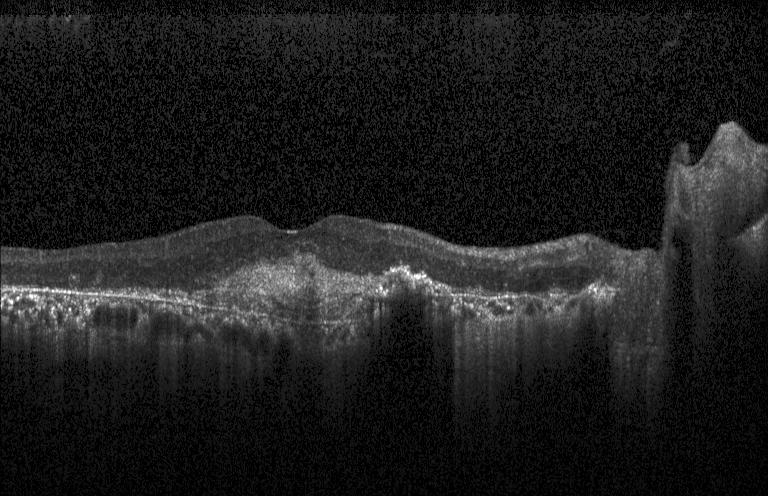 Centered on the fovea, OCT B-scan.
Impression: CNV.